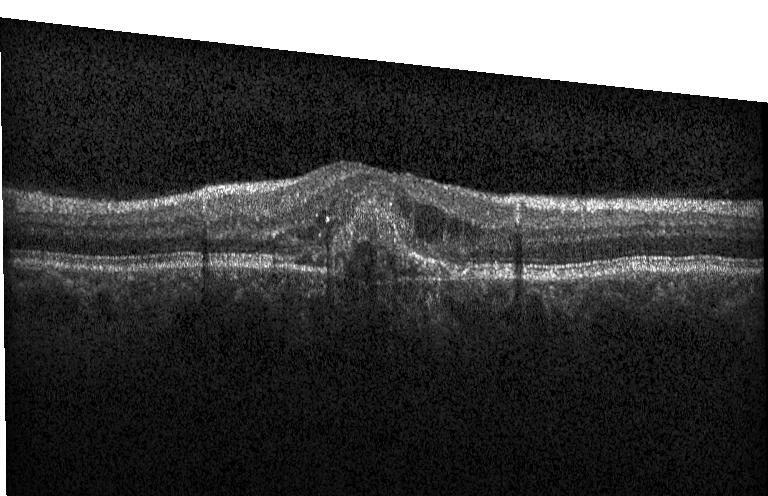 Fovea-centered · spectral-domain OCT · OCT B-scan · acquired on a Heidelberg Spectralis
Dx: a choroidal neovascular membrane.